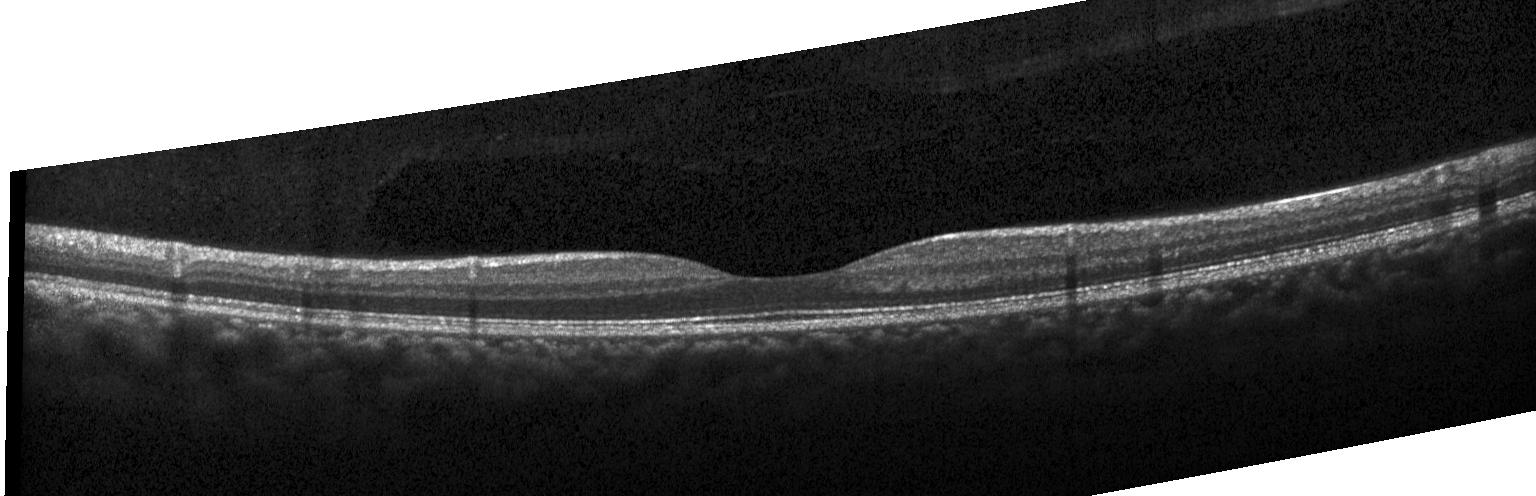

OCT scan showing no choroidal neovascularization, diabetic macular edema, or drusen.